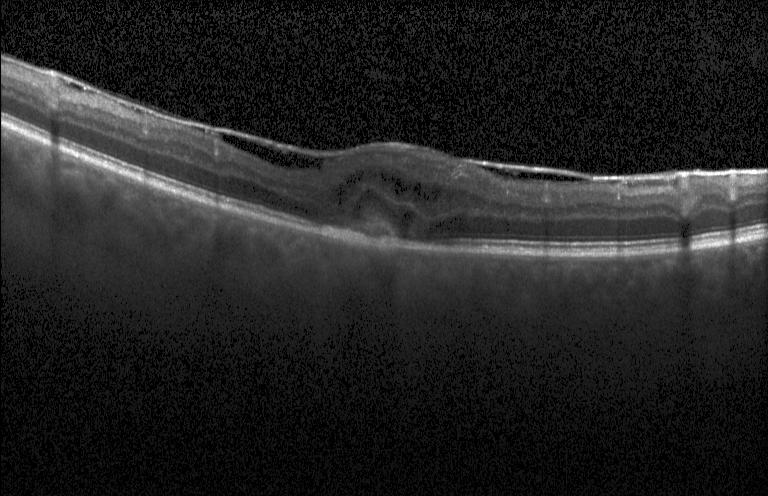 Spectral-domain optical coherence tomography · macular scan · Heidelberg Spectralis OCT system · retinal OCT cross-section. OCT finding: a choroidal neovascular membrane.